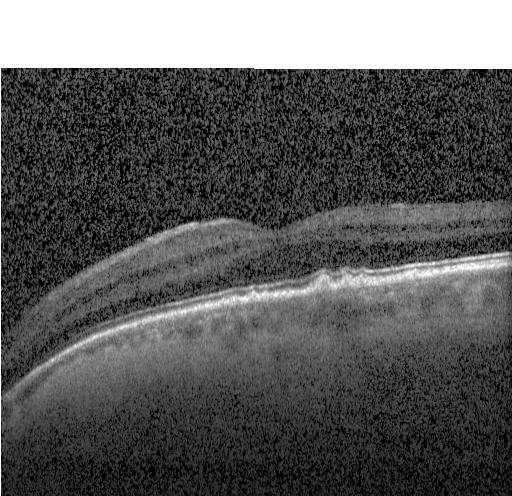
Retinal OCT B-scan. This B-scan demonstrates sub-RPE drusenoid deposits.